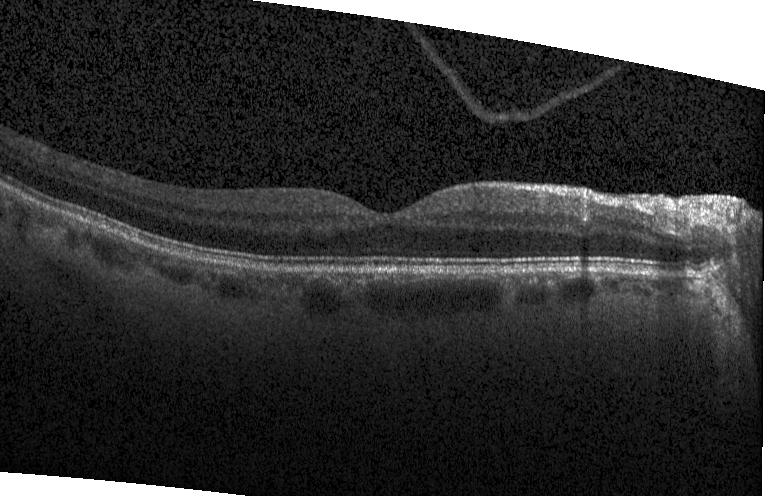

This B-scan demonstrates no CNV, DME, or drusen.